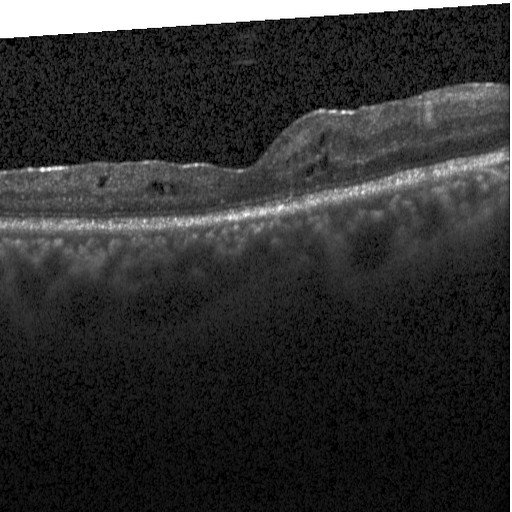
OCT scan showing diabetic macular edema (DME).